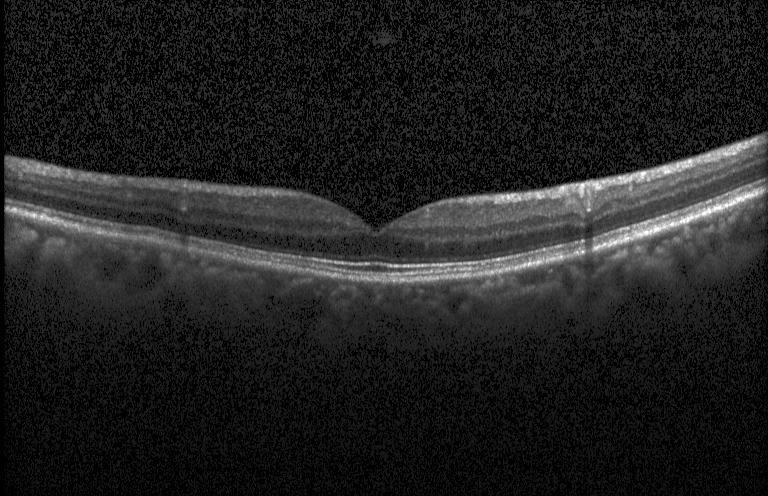 Optical coherence tomography scan. Instrument: Heidelberg Spectralis. Macular scan. Finding: no CNV, DME, or drusen.